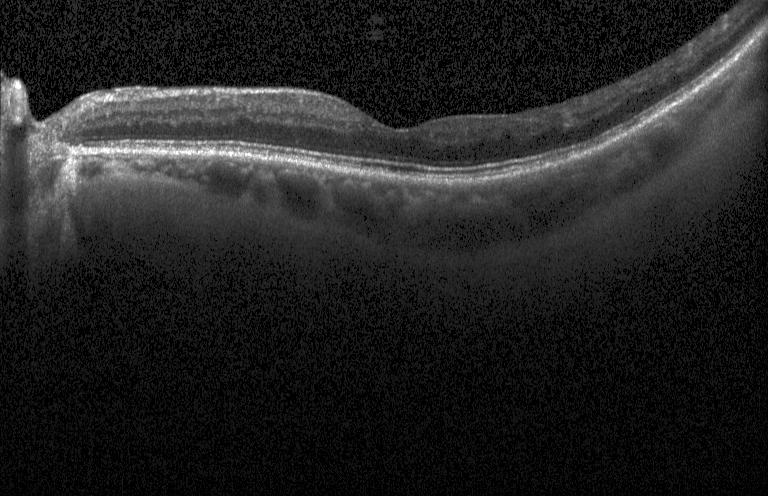

Retinal OCT cross-section; instrument: Heidelberg Spectralis; spectral-domain optical coherence tomography; through the macula
No evidence of choroidal neovascularization, diabetic macular edema, or drusen.